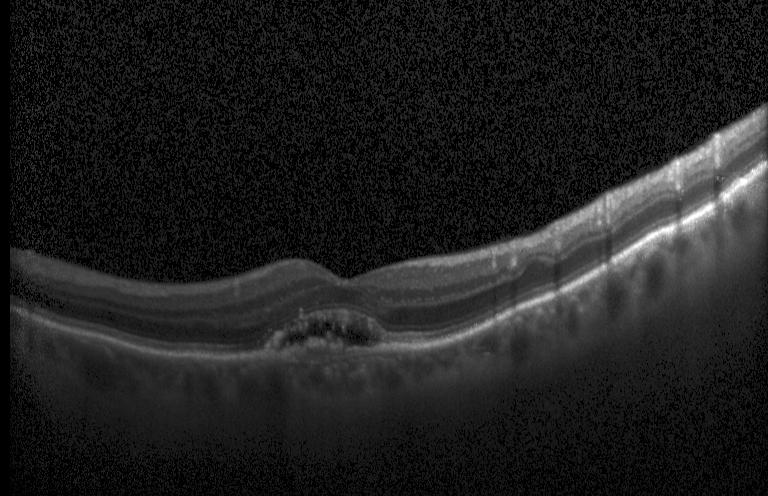

OCT B-scan; spectral-domain OCT; macular scan; Heidelberg Spectralis OCT system — OCT finding: a choroidal neovascular membrane.